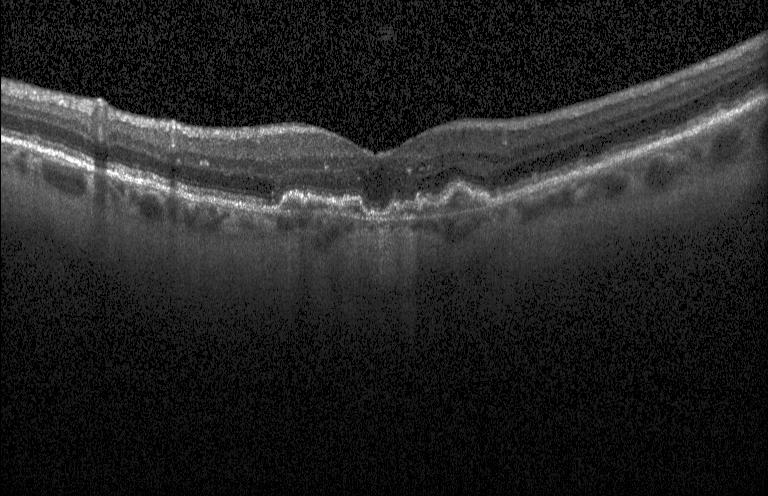

Fovea-centered, OCT B-scan, spectral-domain OCT
This B-scan demonstrates choroidal neovascularization (CNV).